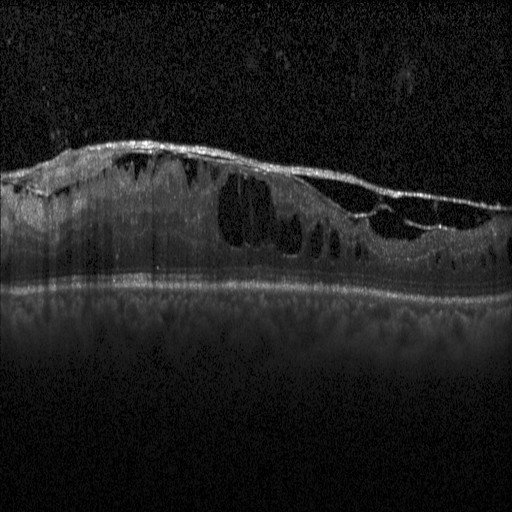 Finding: DME.